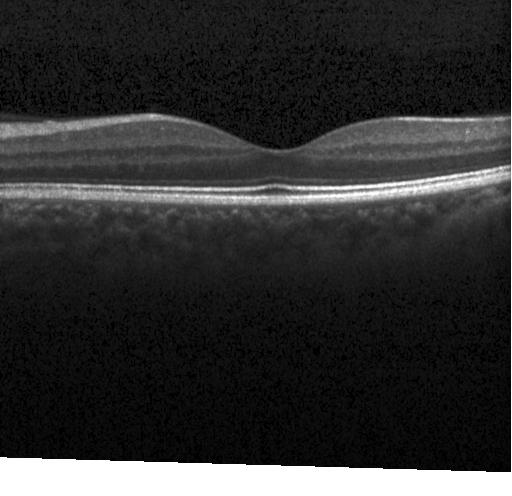 Optical coherence tomography scan. Assessment: no choroidal neovascularization, diabetic macular edema, or drusen.